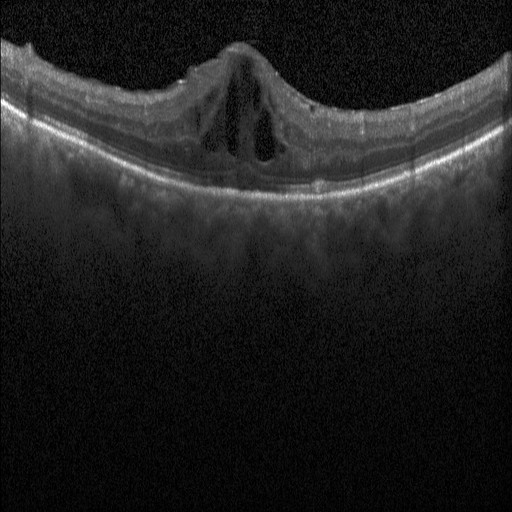 Through the macula, SD-OCT, retinal OCT B-scan. The scan shows diabetic macular edema (DME).